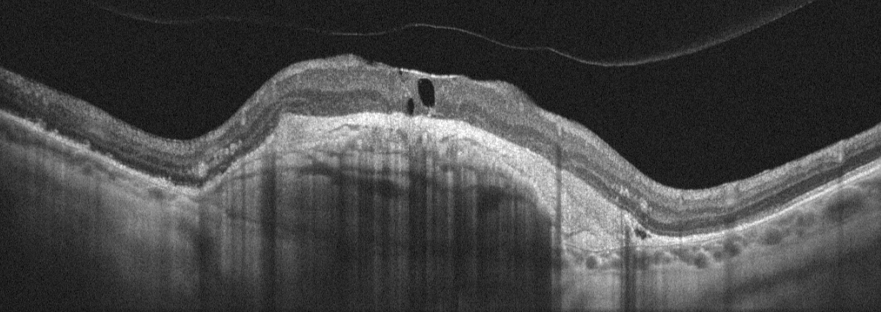
Optovue Avanti RTVue XR. Retinal OCT cross-section. Fovea-centered. Diagnosis: age-related macular degeneration.